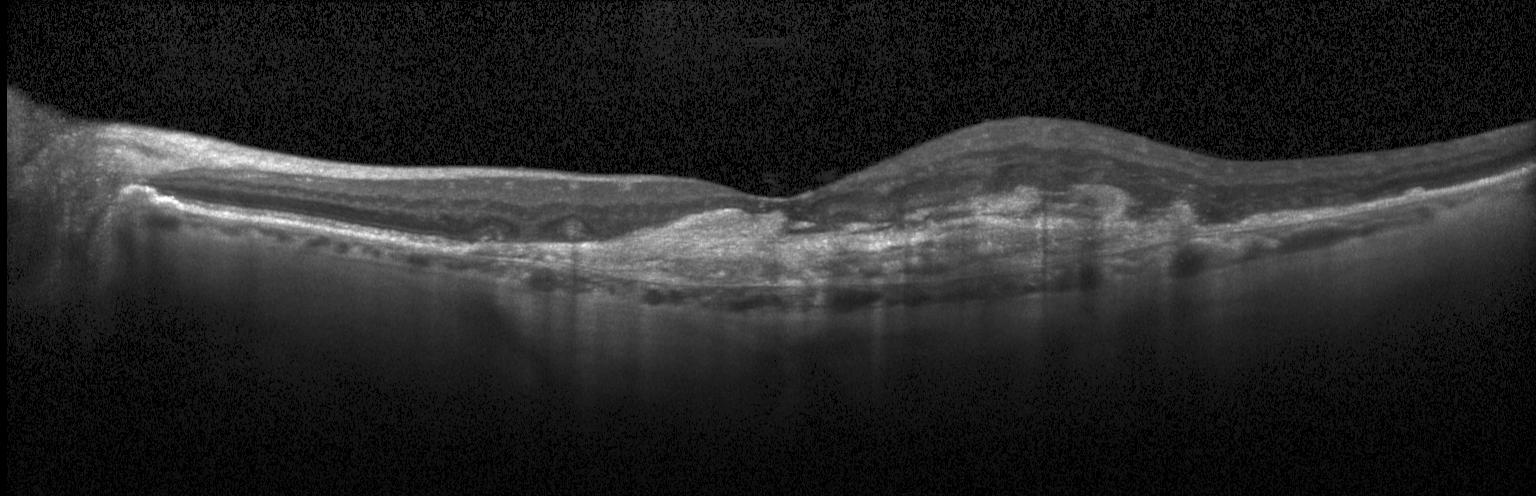 This B-scan demonstrates a choroidal neovascular membrane.